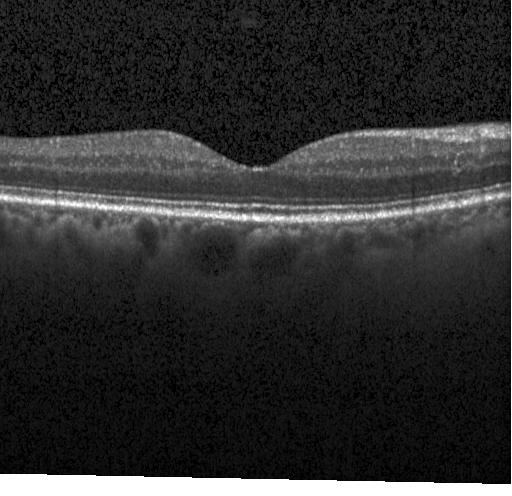

Fovea-centered. Spectral-domain optical coherence tomography. Retinal OCT B-scan — This B-scan demonstrates no CNV, DME, or drusen.